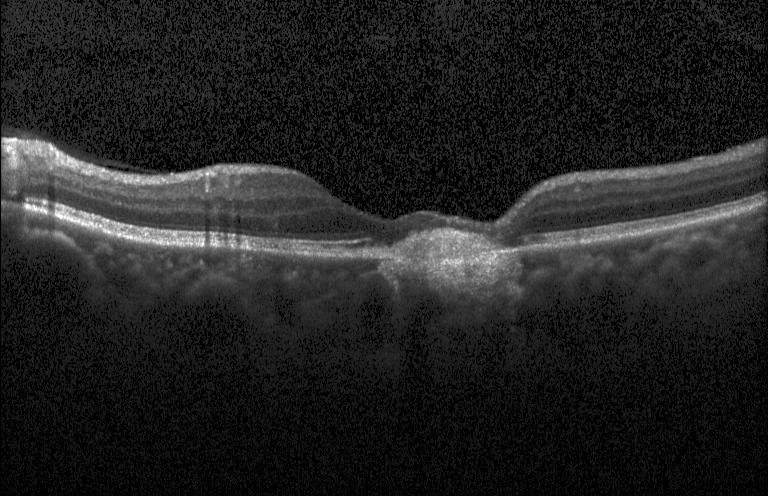 Spectral-domain OCT. Retinal OCT B-scan.
Dx: a choroidal neovascular membrane.